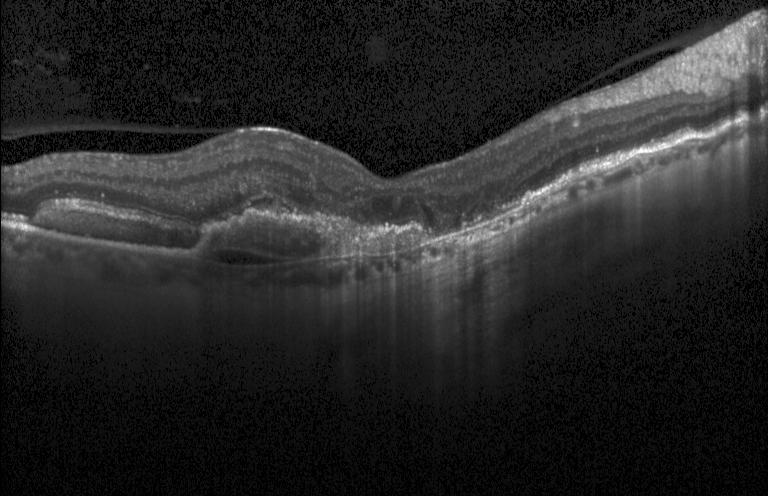 Assessment: a choroidal neovascular membrane.